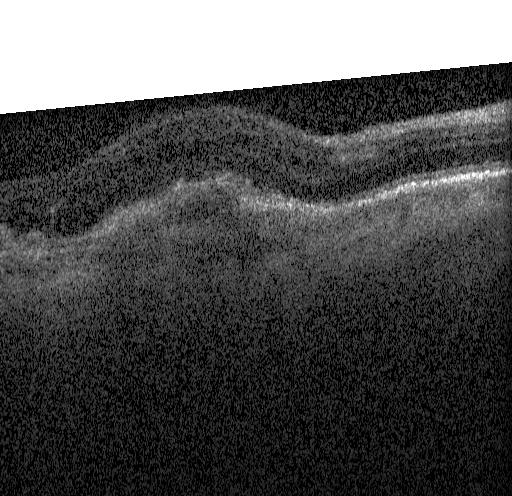 Horizontal scan through the fovea. Heidelberg Spectralis. OCT line scan. Spectral-domain OCT
Diagnosis: a choroidal neovascular membrane.